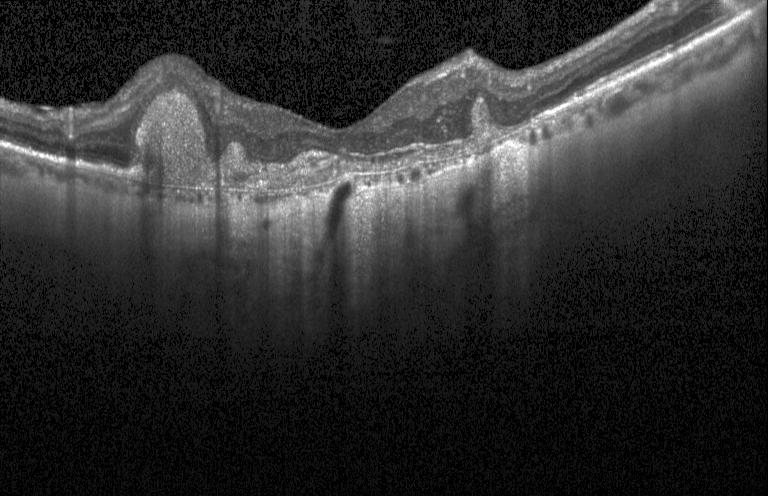
Retinal OCT cross-section — Finding: CNV.